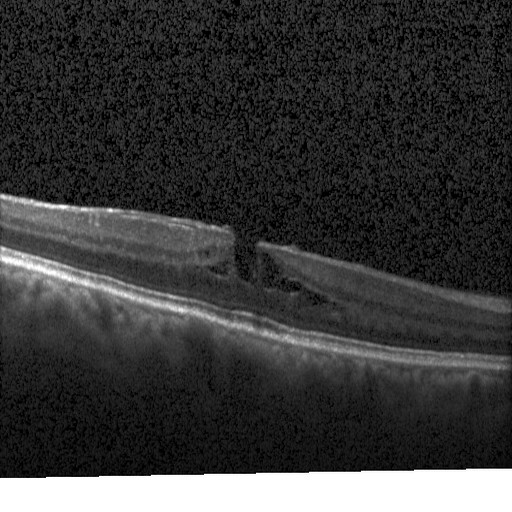
Optical coherence tomography scan — Impression: DME.